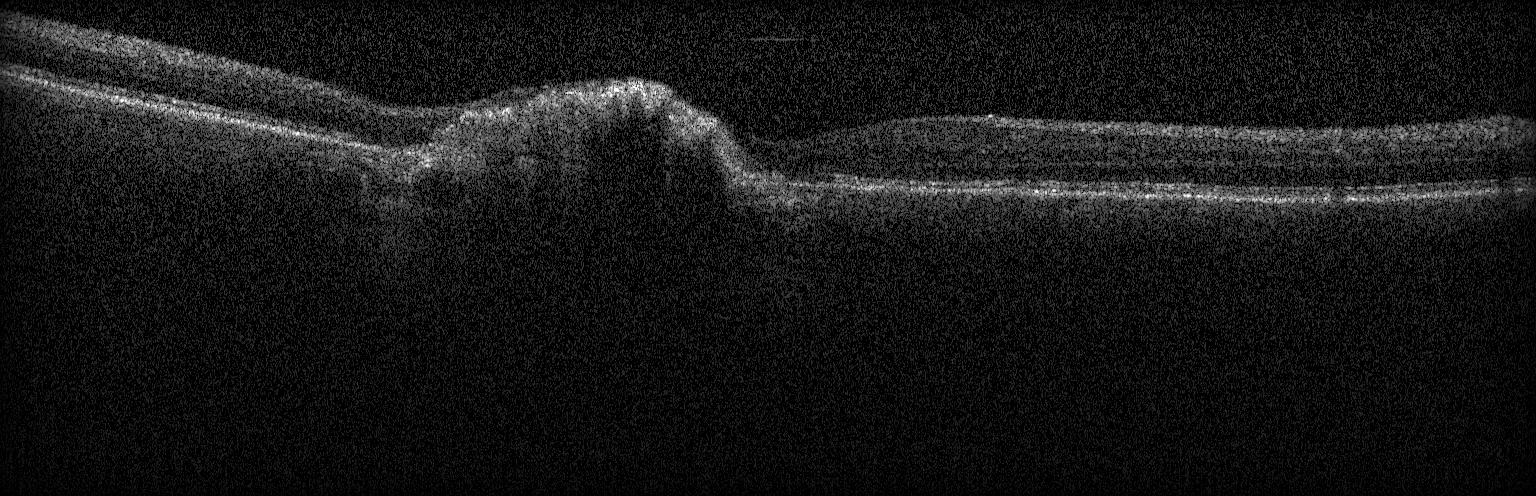

Impression: CNV.